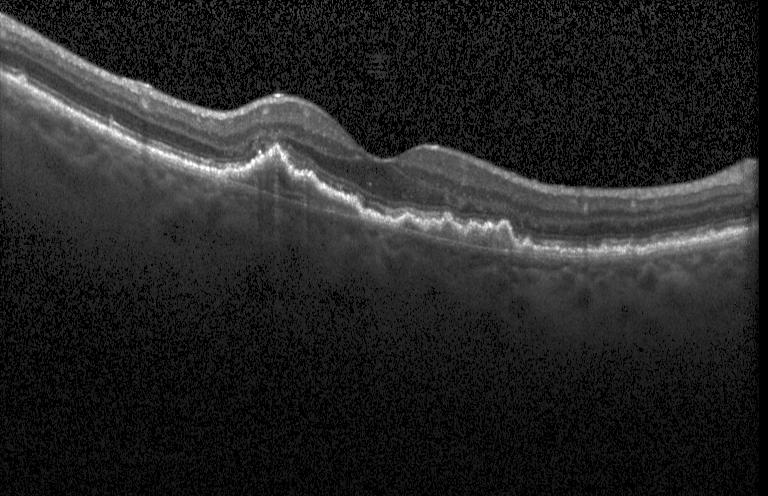

This B-scan demonstrates CNV.